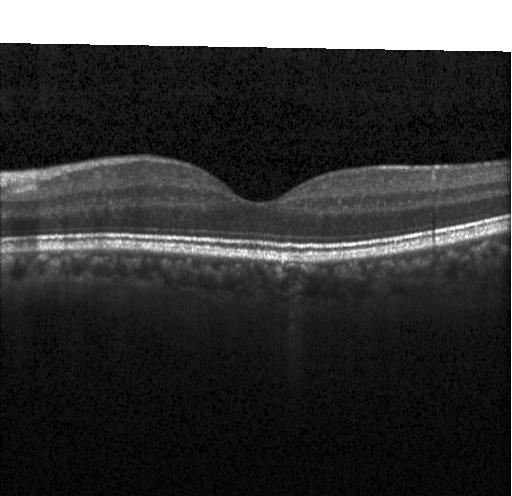 Instrument: Heidelberg Spectralis. Centered on the fovea. Optical coherence tomography scan.
No CNV, DME, or drusen.